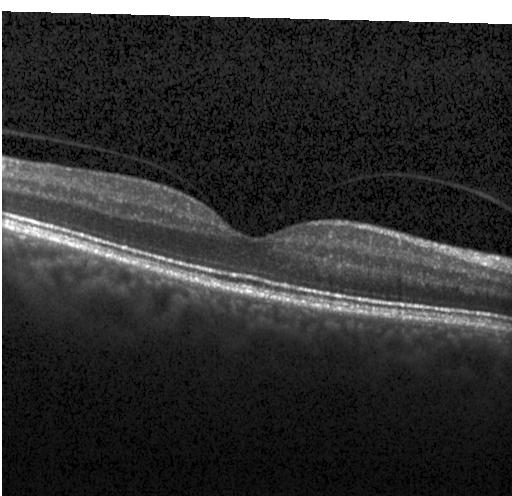 Impression: no evidence of choroidal neovascularization, diabetic macular edema, or drusen.